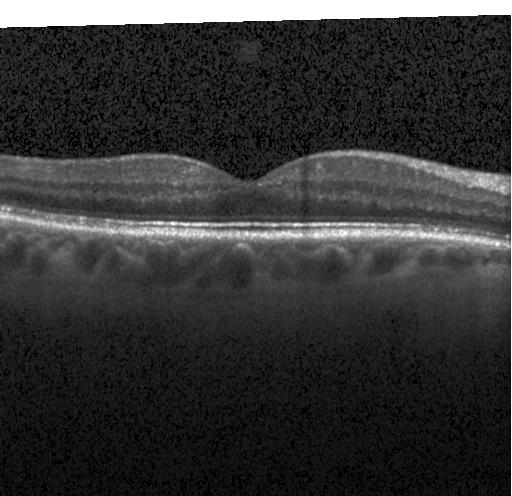 This B-scan demonstrates neither choroidal neovascularization, diabetic macular edema, nor drusen.